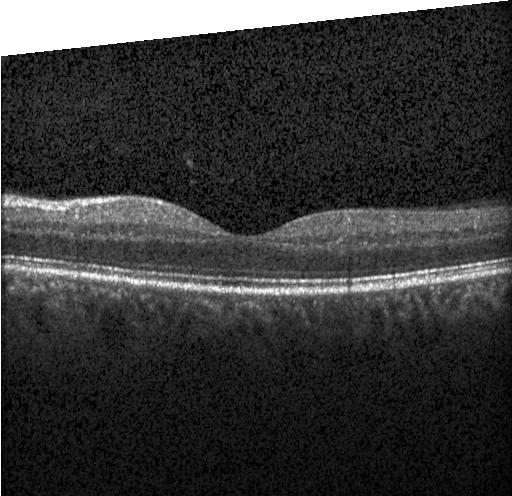
The scan shows neither choroidal neovascularization, diabetic macular edema, nor drusen.